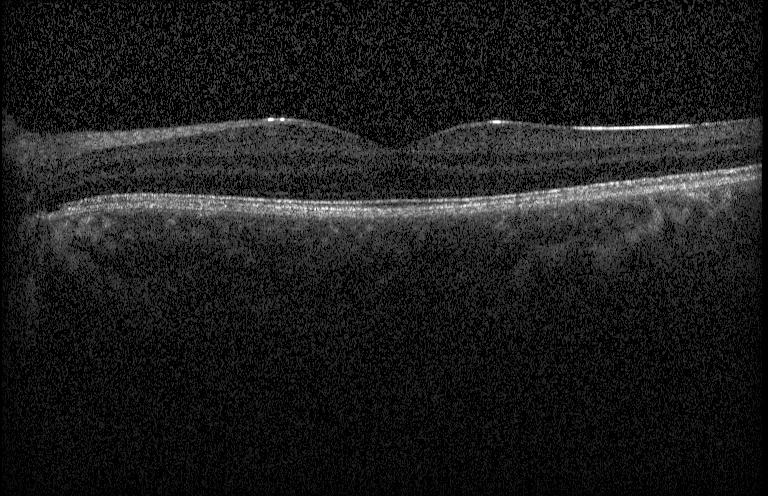 Centered on the fovea; spectral-domain optical coherence tomography; acquired on a Heidelberg Spectralis; optical coherence tomography scan. OCT finding: no choroidal neovascularization, diabetic macular edema, or drusen.